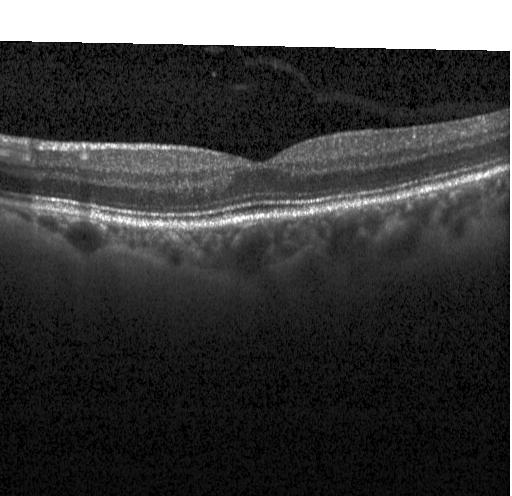
Heidelberg Spectralis; optical coherence tomography scan; spectral-domain optical coherence tomography; fovea-centered — Impression: no choroidal neovascularization, diabetic macular edema, or drusen.